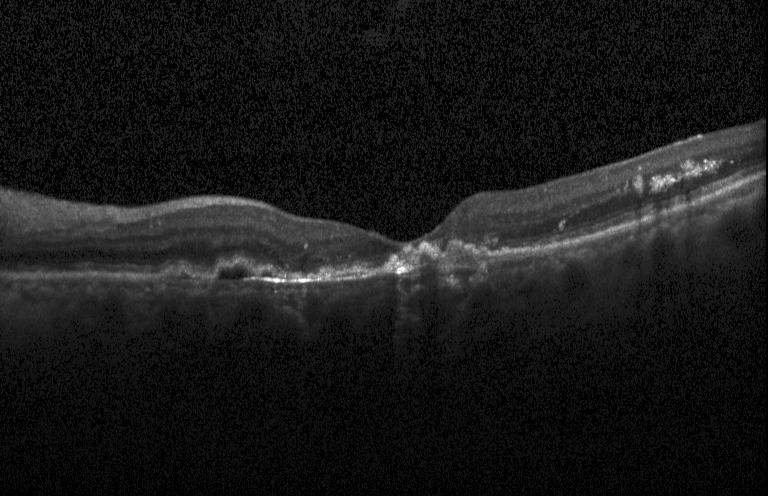 Finding: choroidal neovascularization.